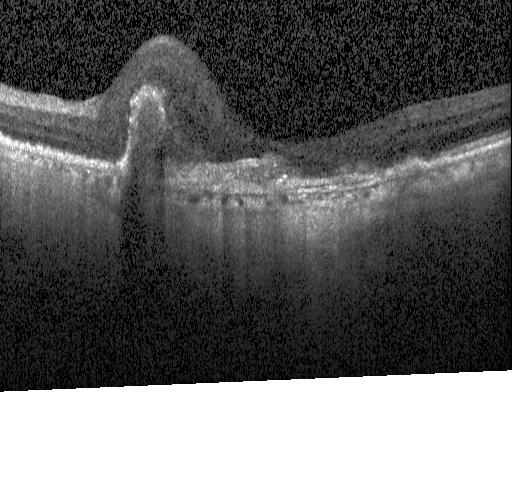 Impression: a choroidal neovascular membrane.